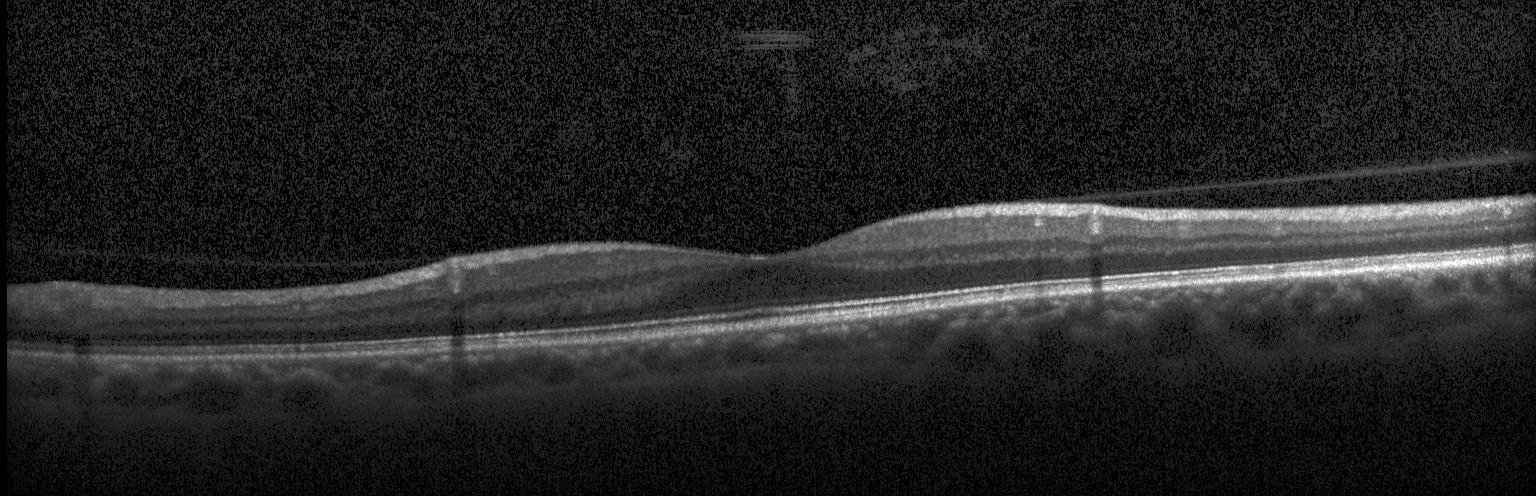 Diagnosis: neither choroidal neovascularization, diabetic macular edema, nor drusen.